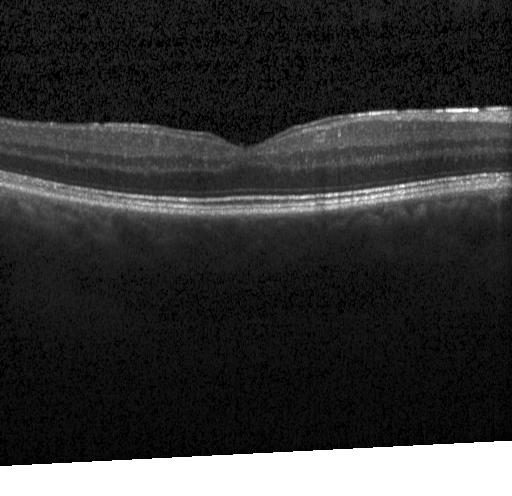 Spectral-domain OCT B-scan: no evidence of choroidal neovascularization, diabetic macular edema, or drusen.